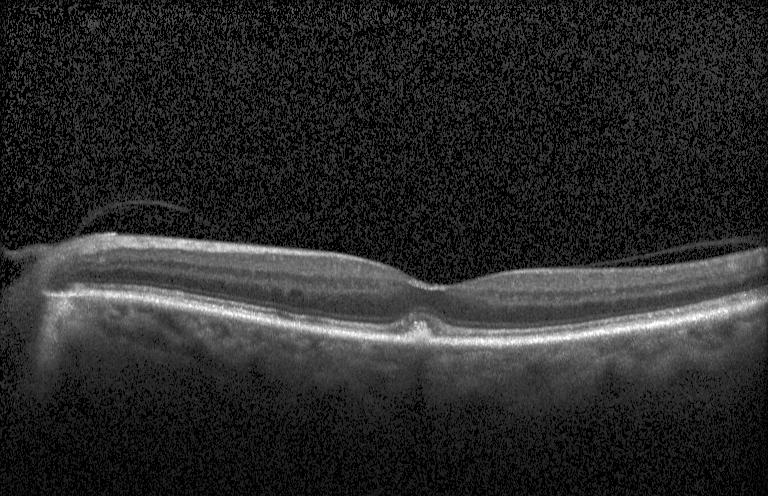 Diagnosis: multiple drusen.